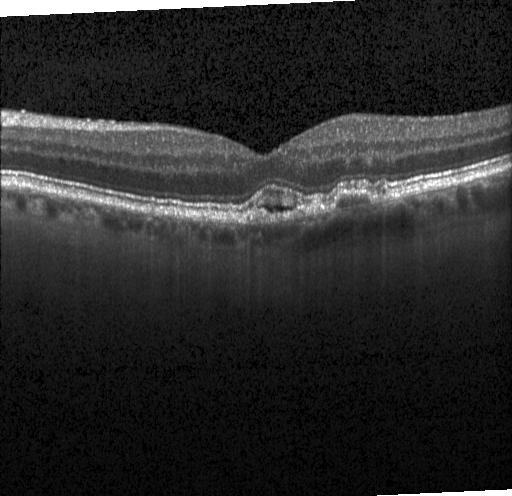
Optical coherence tomography B-scan, spectral-domain optical coherence tomography, acquired on a Heidelberg Spectralis.
Finding: CNV.